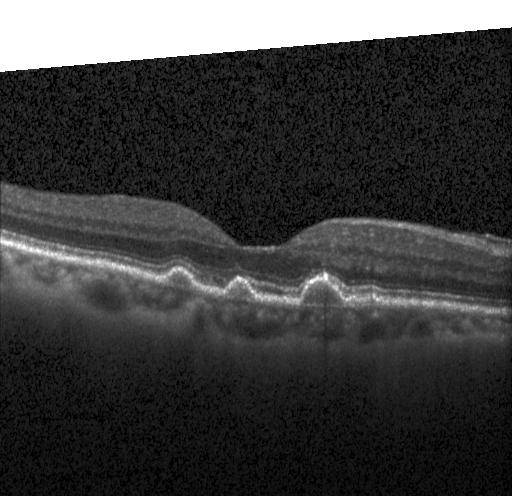 Multiple drusen.